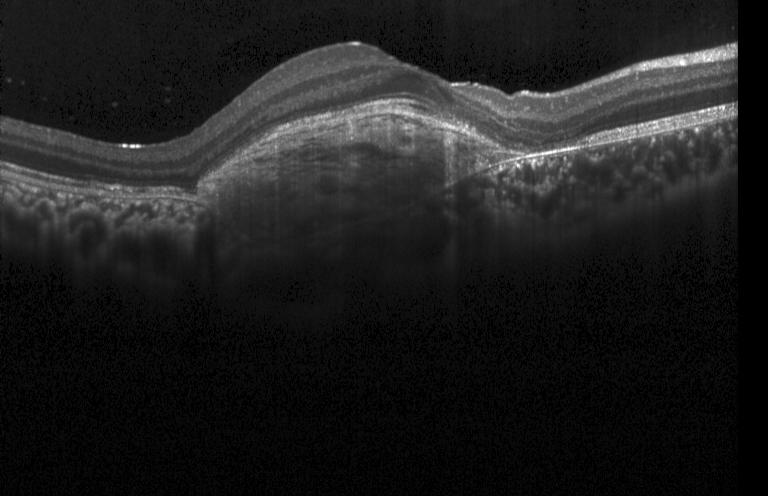
Macular scan; spectral-domain OCT; retinal OCT B-scan; Heidelberg Spectralis. Diagnosis: a choroidal neovascular membrane.